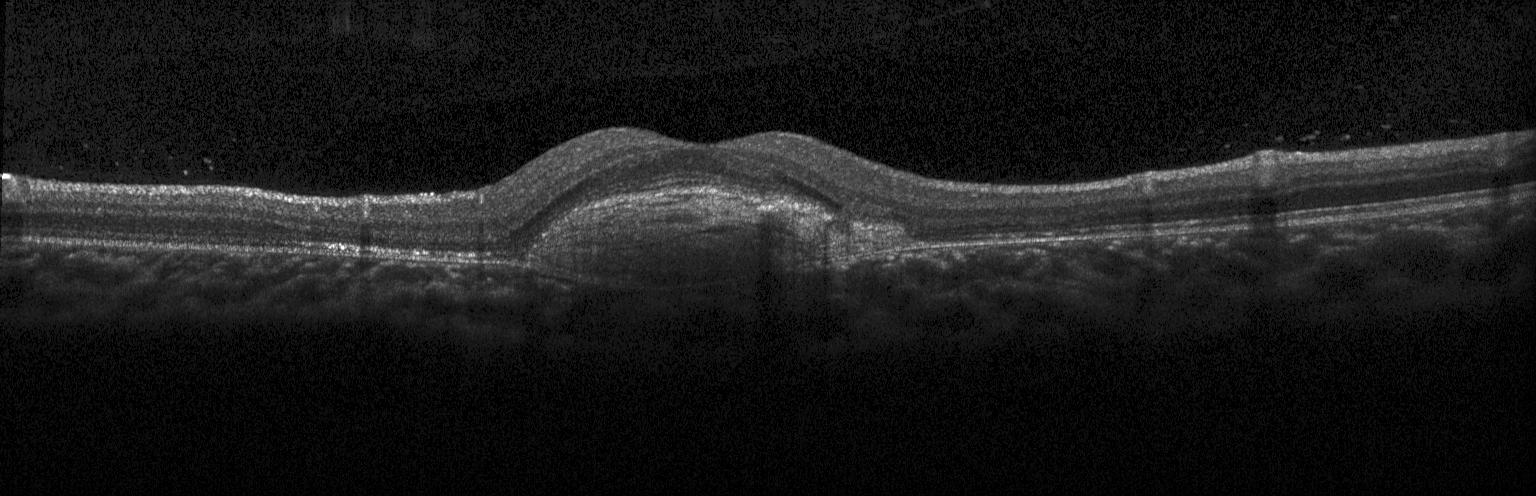
Horizontal scan through the fovea. Heidelberg Spectralis. OCT B-scan.
Diagnosis: a choroidal neovascular membrane.